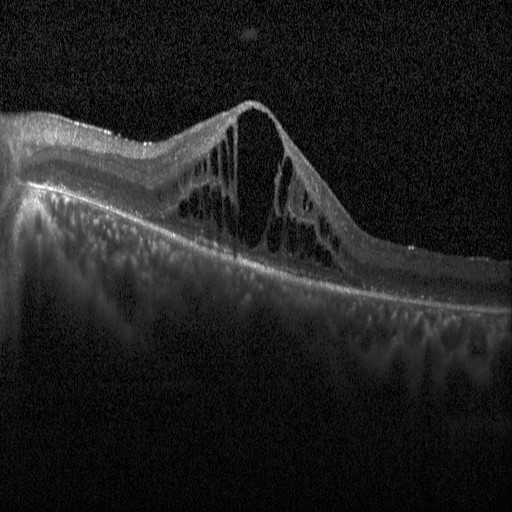 Dx: DME.